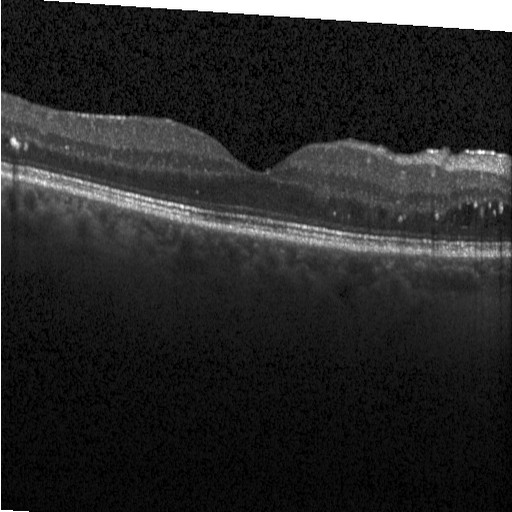
Fovea-centered · retinal OCT B-scan. The scan shows DME.